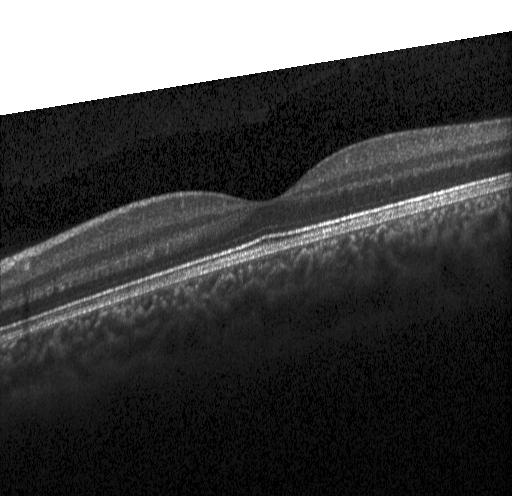 Retinal OCT cross-section. Macular scan. Instrument: Heidelberg Spectralis. Impression: no choroidal neovascularization, diabetic macular edema, or drusen.